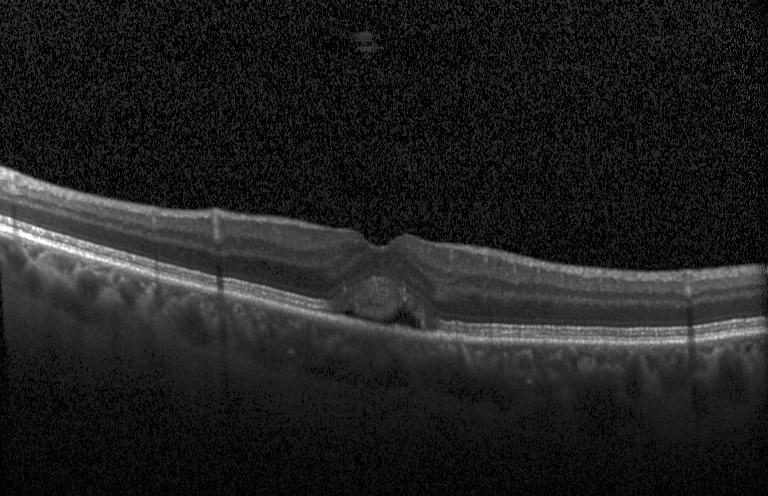 Macular OCT demonstrating CNV.